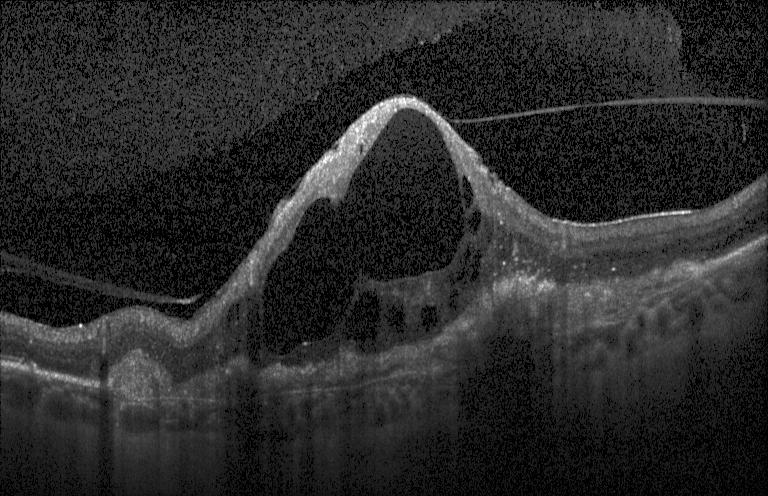 Through the macula. Optical coherence tomography B-scan.
Diagnosis: a choroidal neovascular membrane.